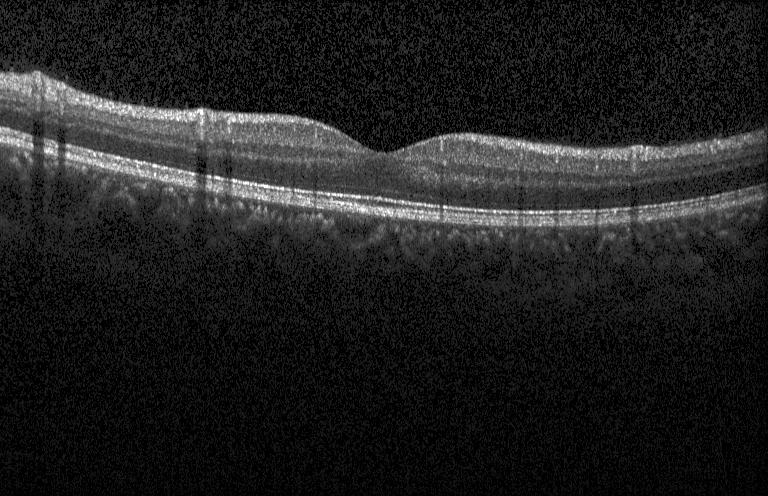 OCT line scan.
Diagnosis: no CNV, DME, or drusen.